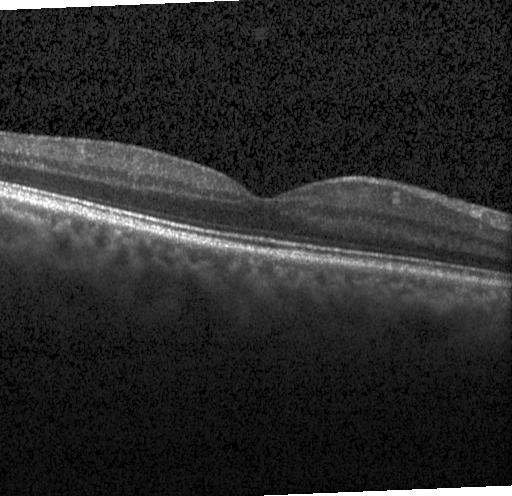 Retinal OCT cross-section. Spectral-domain OCT. Through the macula. Heidelberg Spectralis OCT system. This B-scan demonstrates no choroidal neovascularization, diabetic macular edema, or drusen.